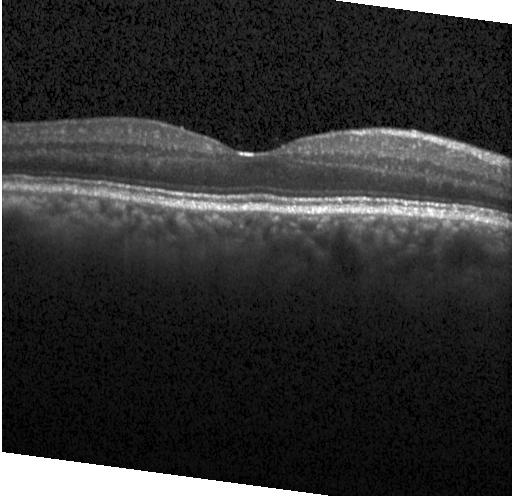

OCT B-scan · centered on the fovea
Diagnosis: no choroidal neovascularization, diabetic macular edema, or drusen.